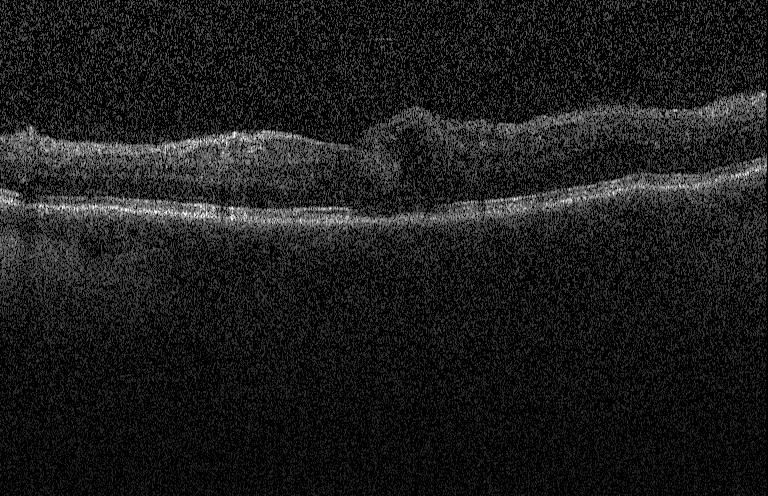 Diagnosis: diabetic macular edema (DME).